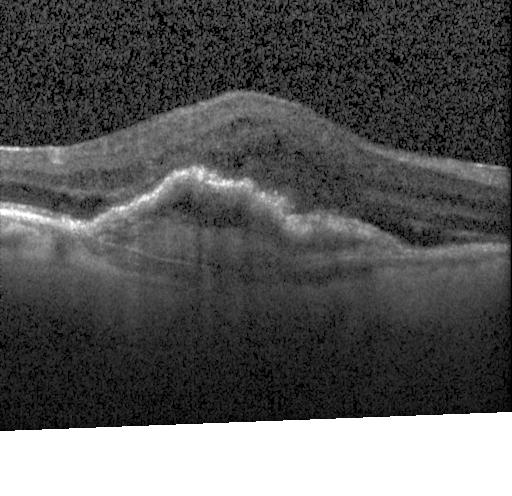 Optical coherence tomography B-scan; SD-OCT
Assessment: choroidal neovascularization (CNV).